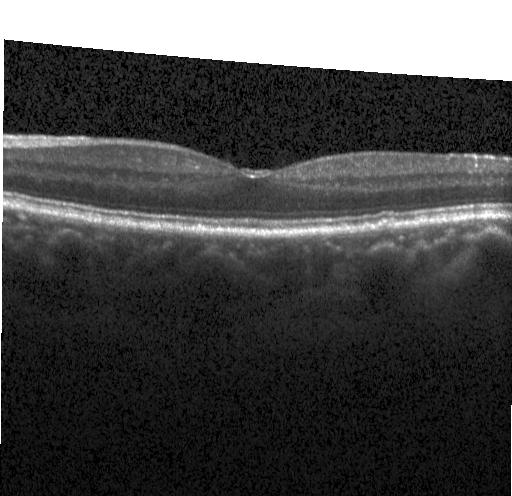
Impression: sub-RPE drusenoid deposits.